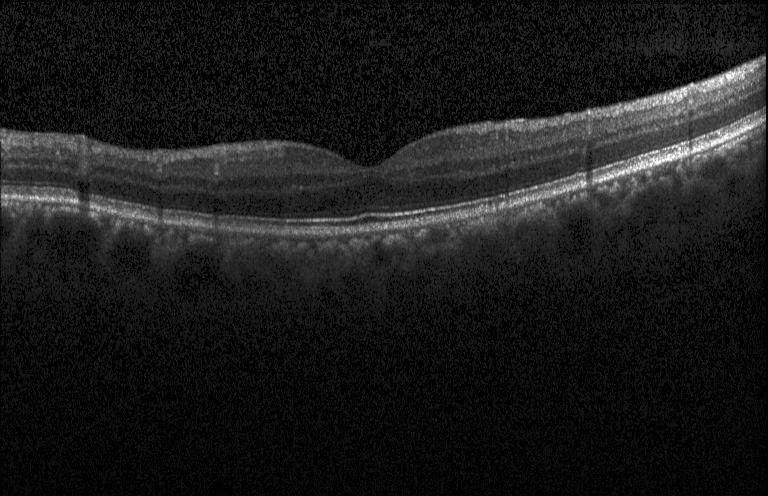
OCT finding: no choroidal neovascularization, diabetic macular edema, or drusen.